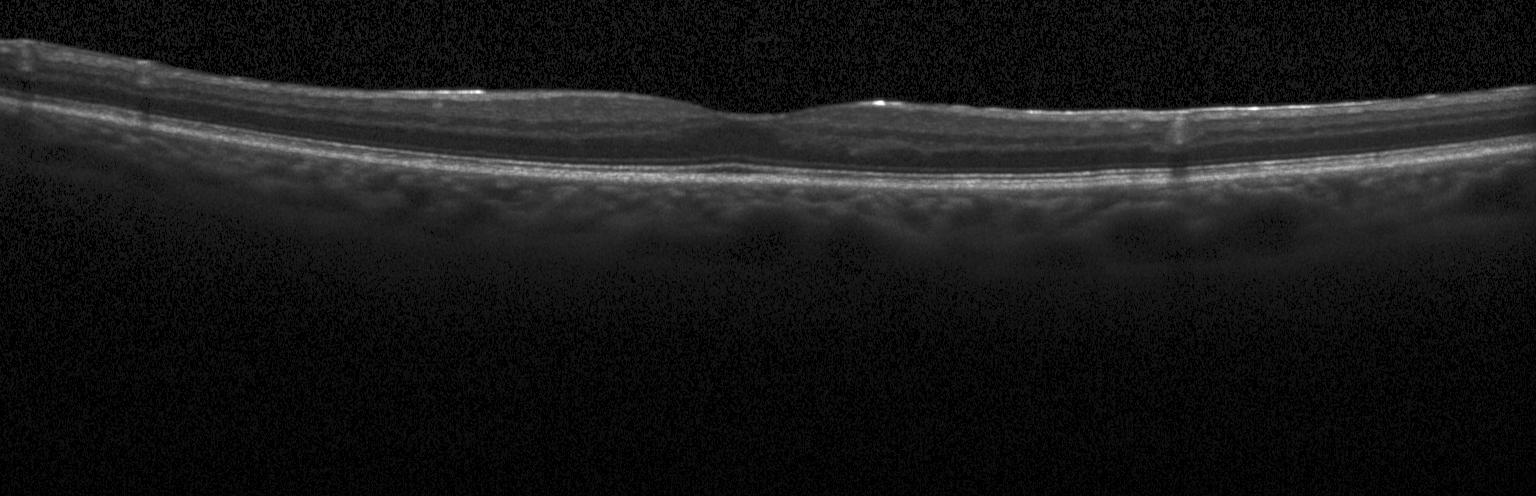

Retinal OCT B-scan; instrument: Heidelberg Spectralis. The scan shows no evidence of choroidal neovascularization, diabetic macular edema, or drusen.